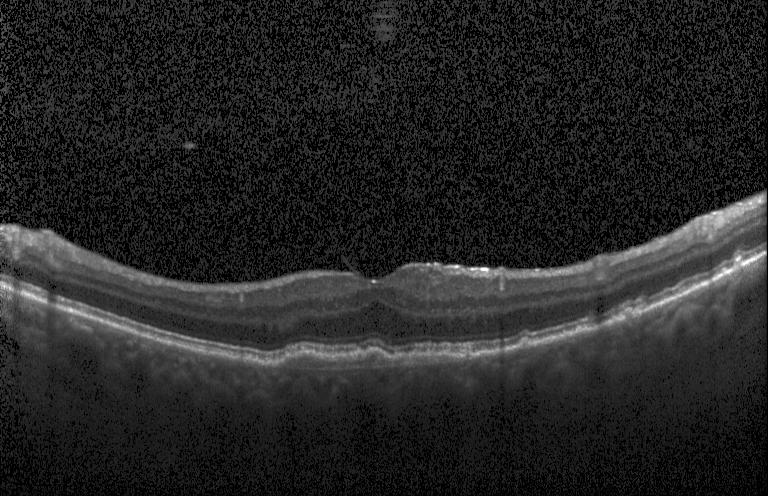

Instrument: Heidelberg Spectralis, OCT B-scan, spectral-domain optical coherence tomography
Assessment: choroidal neovascularization.